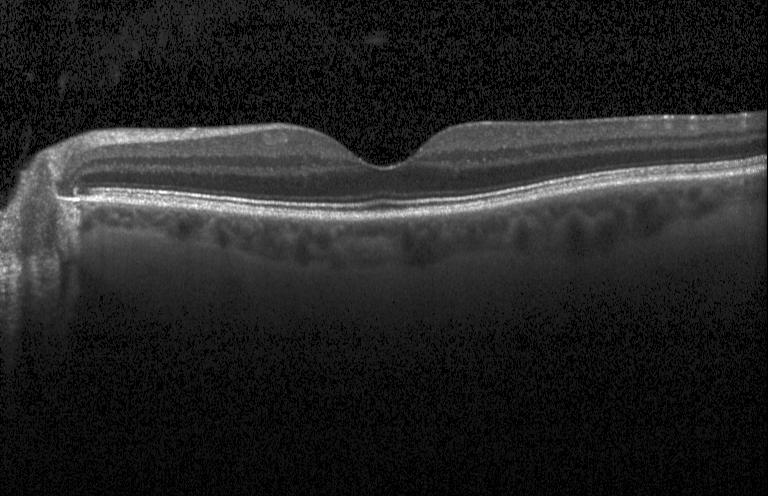

OCT finding: no CNV, DME, or drusen.